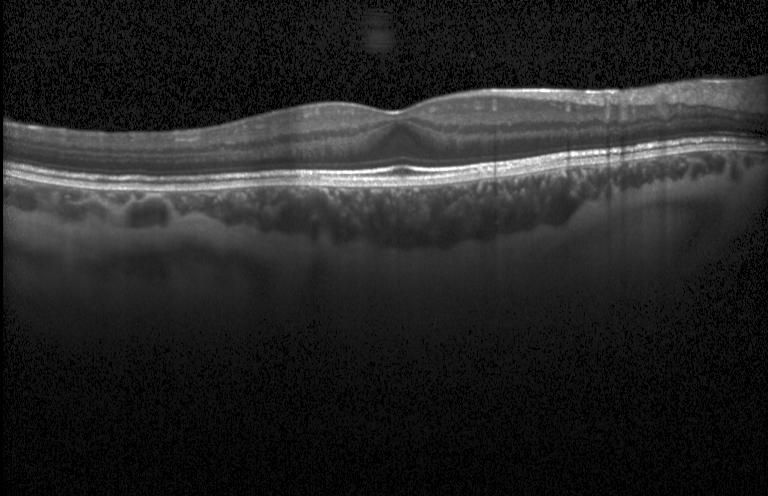 Diagnosis: no CNV, DME, or drusen.